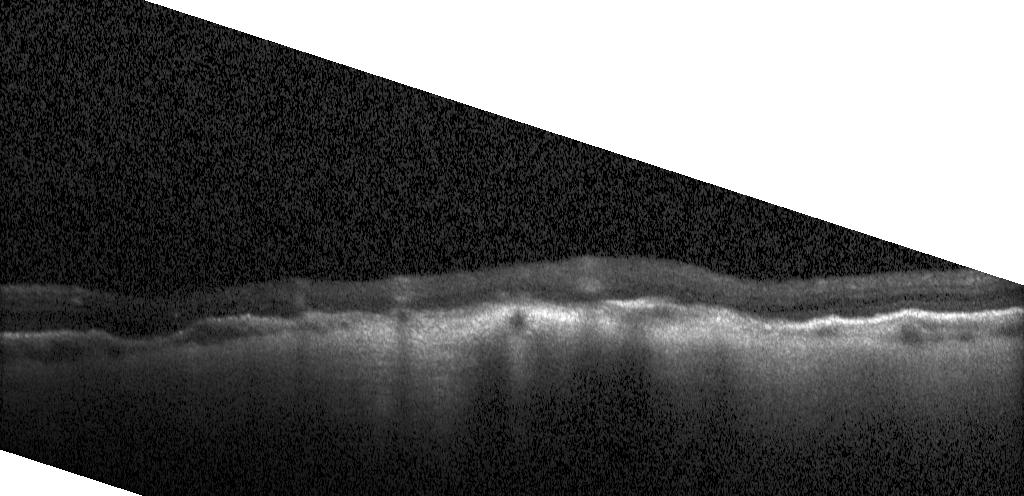 SD-OCT; optical coherence tomography scan — Impression: a choroidal neovascular membrane.